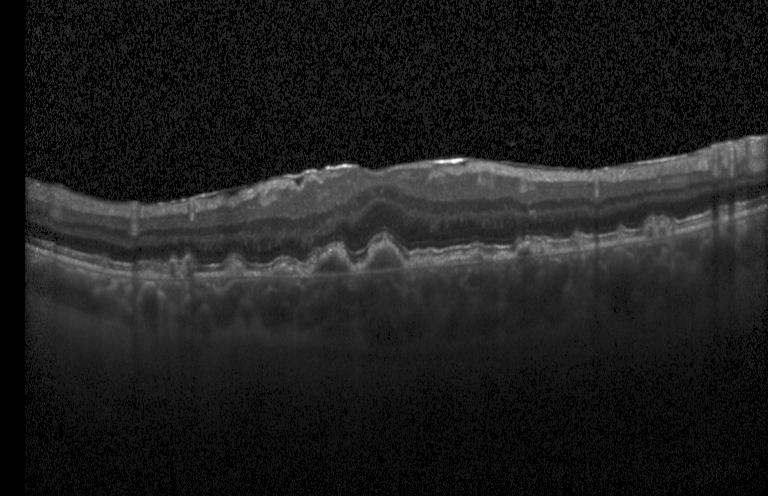
Impression: a choroidal neovascular membrane.